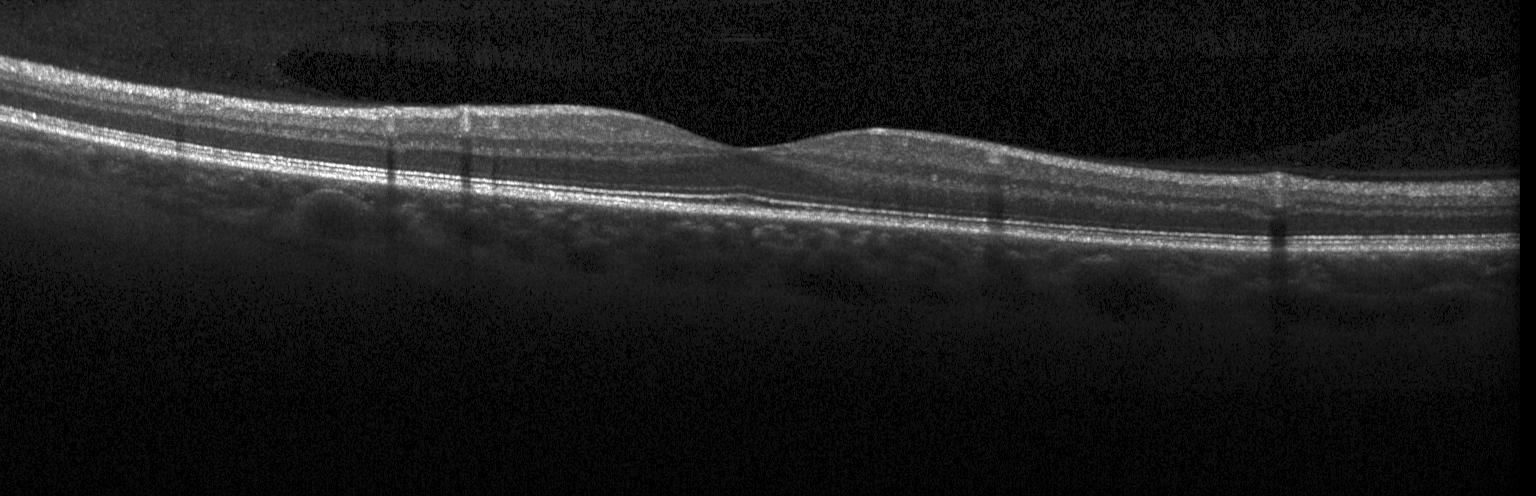

OCT line scan.
This B-scan demonstrates no choroidal neovascularization, no diabetic macular edema, and no drusen.